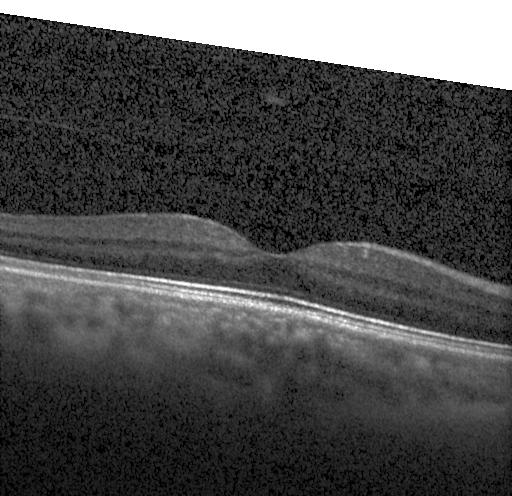 Macular OCT demonstrating no choroidal neovascularization, no diabetic macular edema, and no drusen.